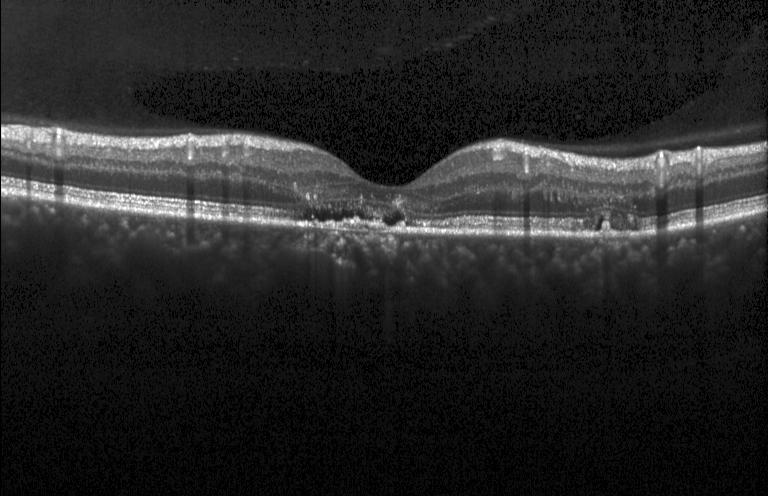

Spectral-domain optical coherence tomography. Retinal OCT B-scan. Centered on the fovea. Instrument: Heidelberg Spectralis
Diagnosis: a choroidal neovascular membrane.